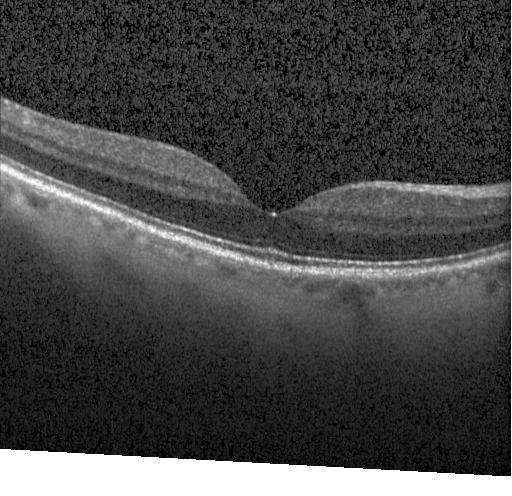

Fovea-centered; optical coherence tomography scan. Diagnosis: neither choroidal neovascularization, diabetic macular edema, nor drusen.